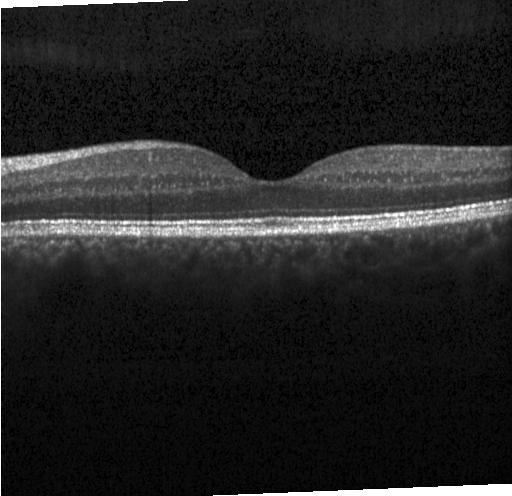
No evidence of CNV, DME, or drusen.